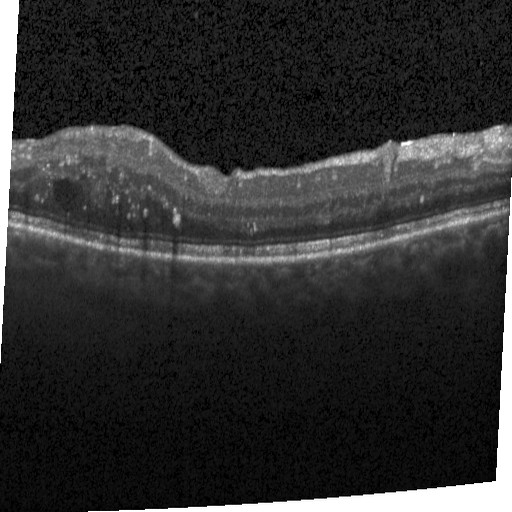 OCT line scan — Dx: DME.